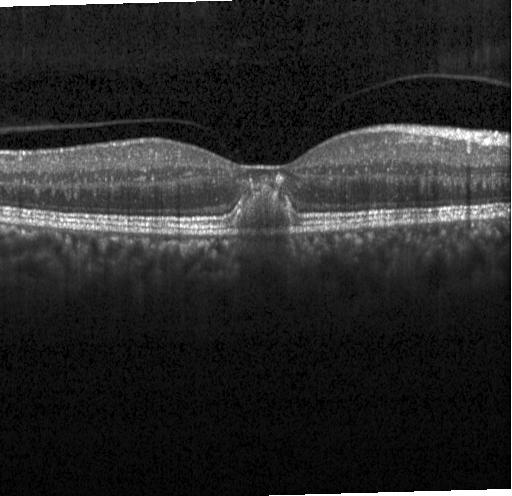
OCT scan showing a choroidal neovascular membrane.